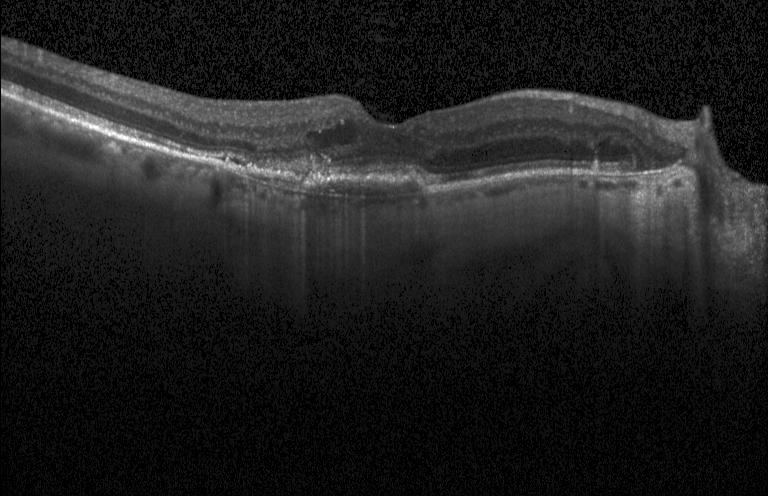

OCT B-scan showing a choroidal neovascular membrane.